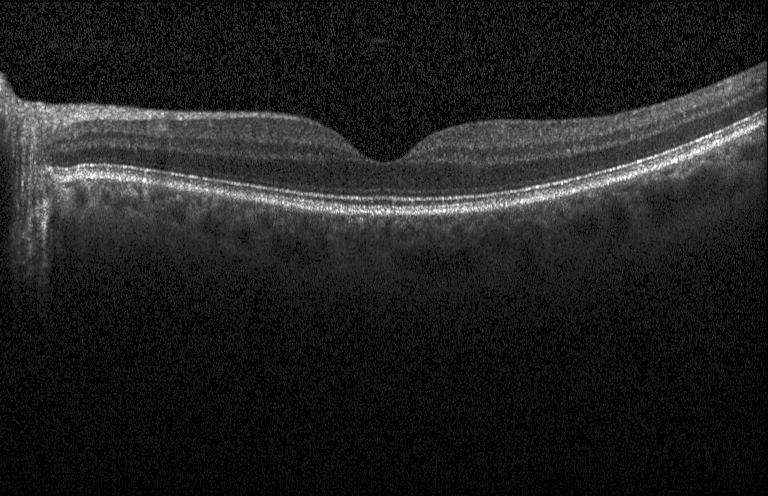

Finding: no CNV, no DME, and no drusen.